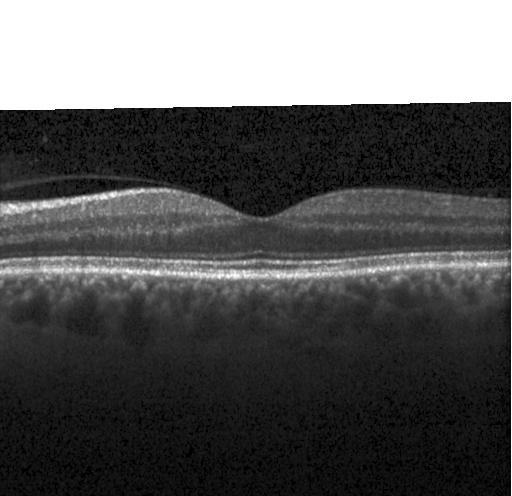
Diagnosis: no evidence of choroidal neovascularization, diabetic macular edema, or drusen.